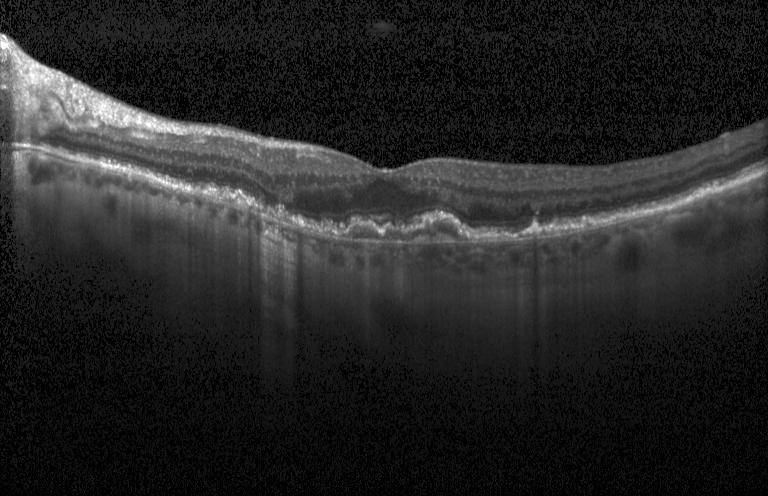 Retinal OCT cross-section showing choroidal neovascularization (CNV).